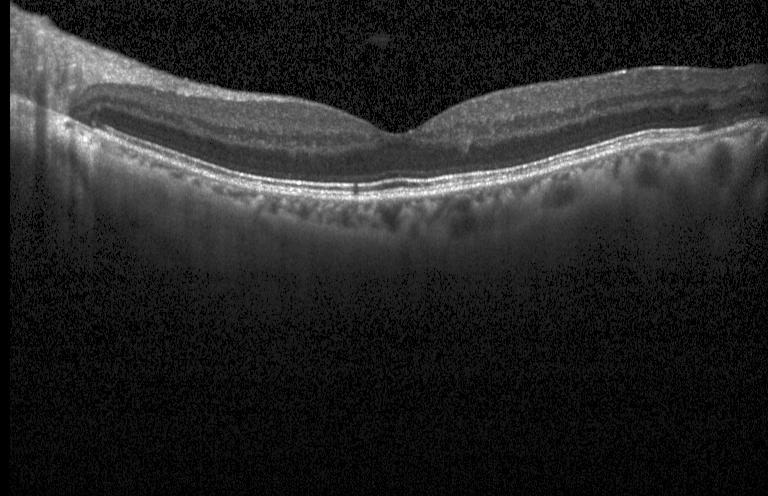

Heidelberg Spectralis; centered on the fovea; optical coherence tomography B-scan. Assessment: no evidence of choroidal neovascularization, diabetic macular edema, or drusen.